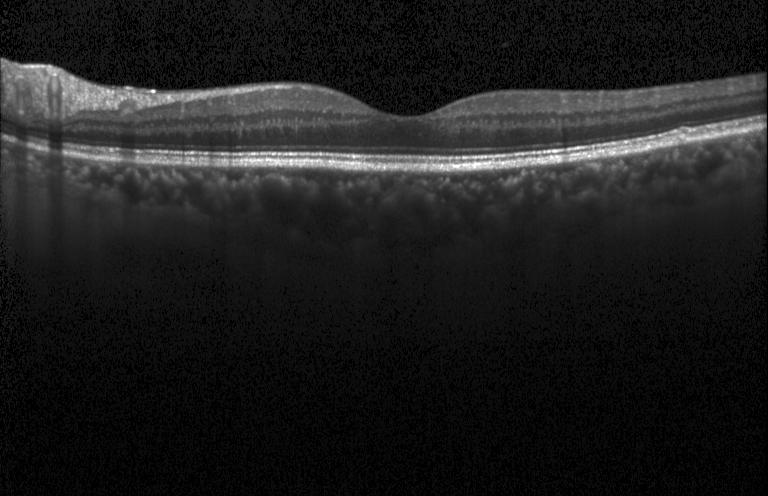 Diagnosis: no evidence of CNV, DME, or drusen.